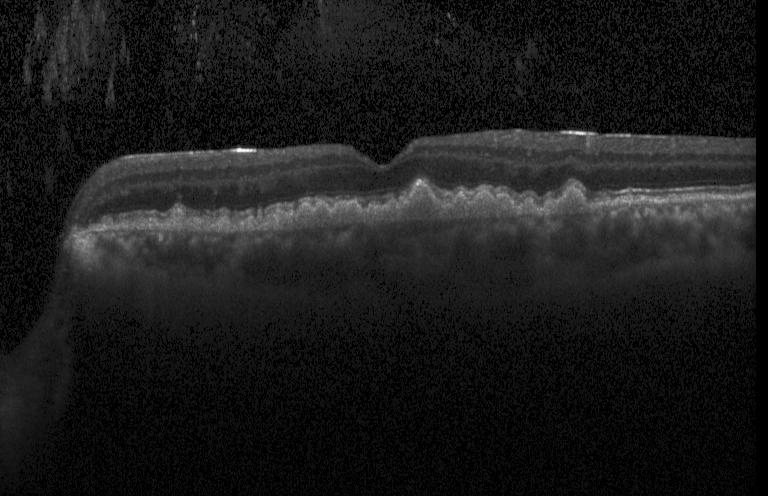
Spectral-domain OCT · Heidelberg Spectralis OCT system · OCT line scan · centered on the fovea.
Finding: a choroidal neovascular membrane.